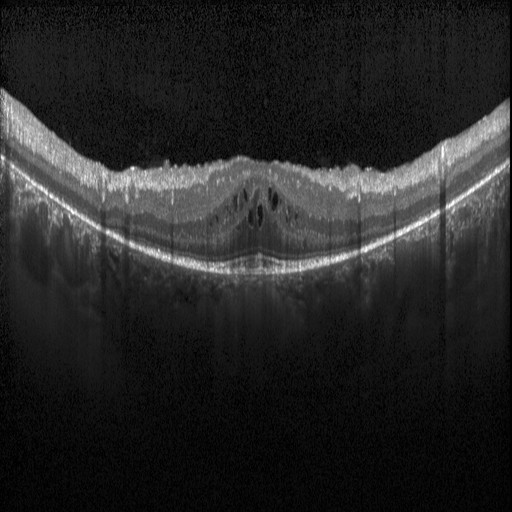 DME.